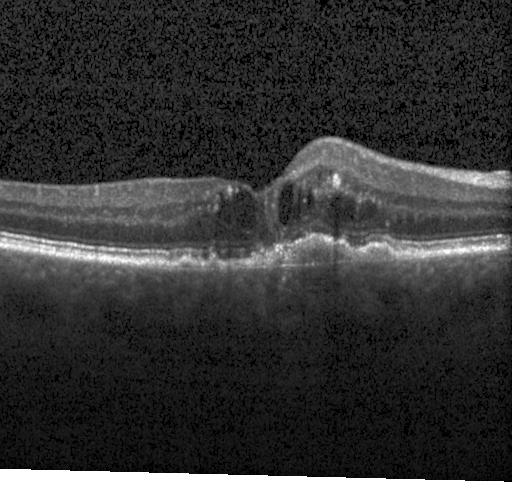
Optical coherence tomography B-scan; SD-OCT.
A choroidal neovascular membrane.